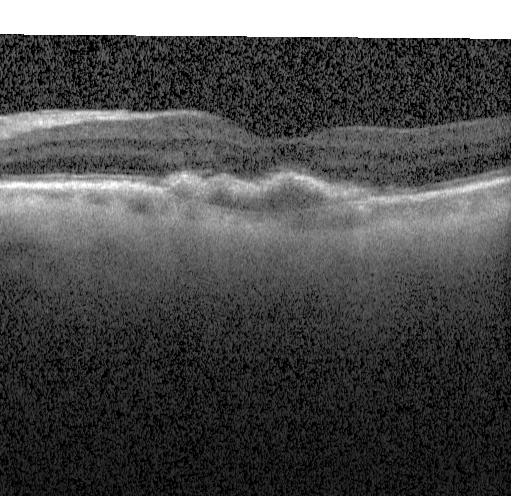 This B-scan demonstrates a choroidal neovascular membrane.